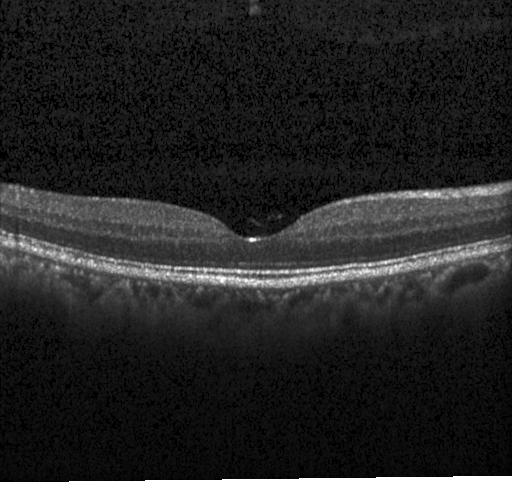 Optical coherence tomography scan
Finding: neither CNV, DME, nor drusen.